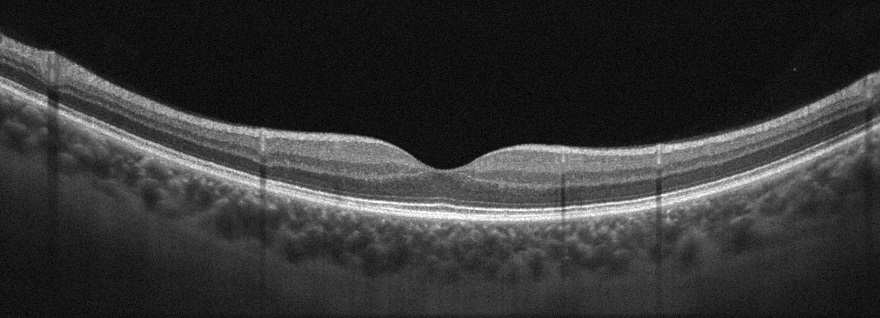

Macular scan, acquired on an Optovue Avanti RTVue XR, optical coherence tomography B-scan.
Finding: no evidence of AMD, DME, ERM, RAO, RVO, or VID.